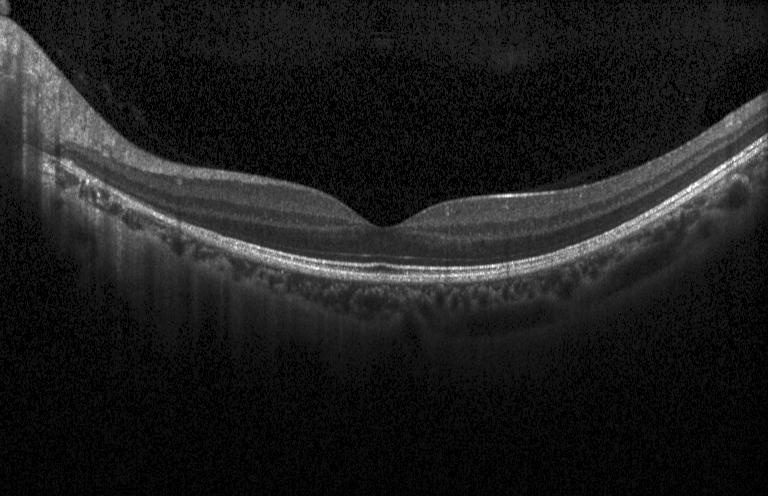
SD-OCT; Heidelberg Spectralis OCT system; OCT B-scan — Assessment: neither choroidal neovascularization, diabetic macular edema, nor drusen.